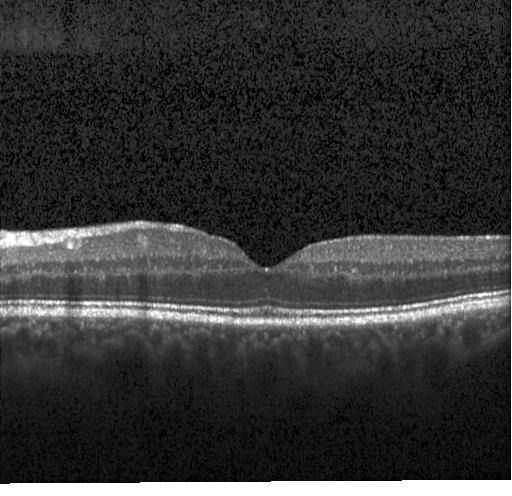 Macular OCT: no choroidal neovascularization, diabetic macular edema, or drusen.